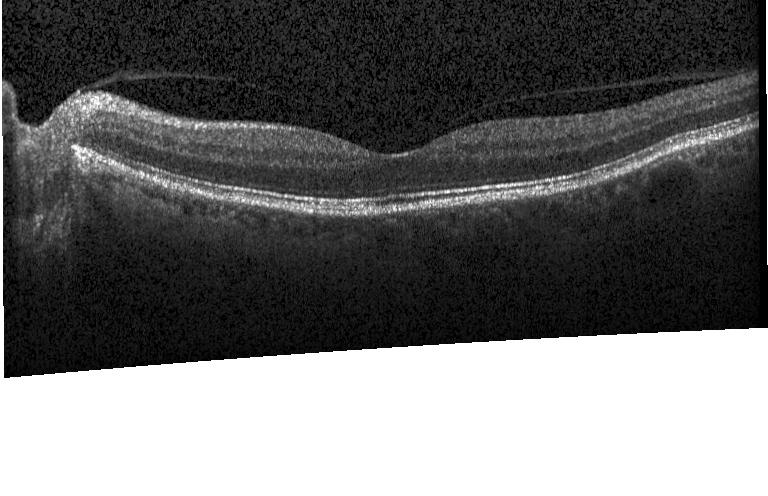
Retinal OCT cross-section — This B-scan demonstrates no choroidal neovascularization, diabetic macular edema, or drusen.